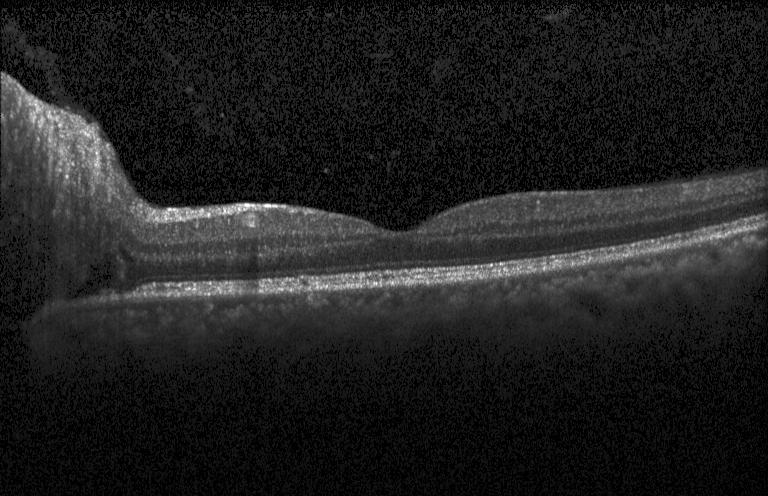 No CNV, DME, or drusen.